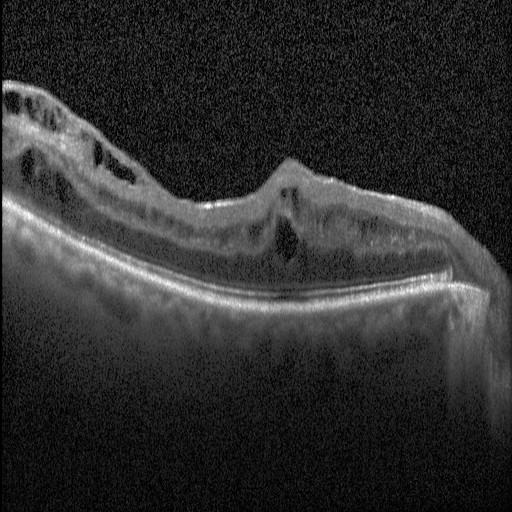 OCT scan showing diabetic macular edema (DME).